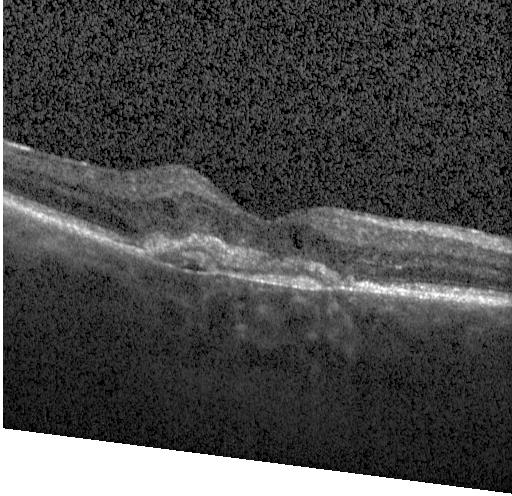
SD-OCT. Retinal OCT cross-section — Impression: choroidal neovascularization (CNV).